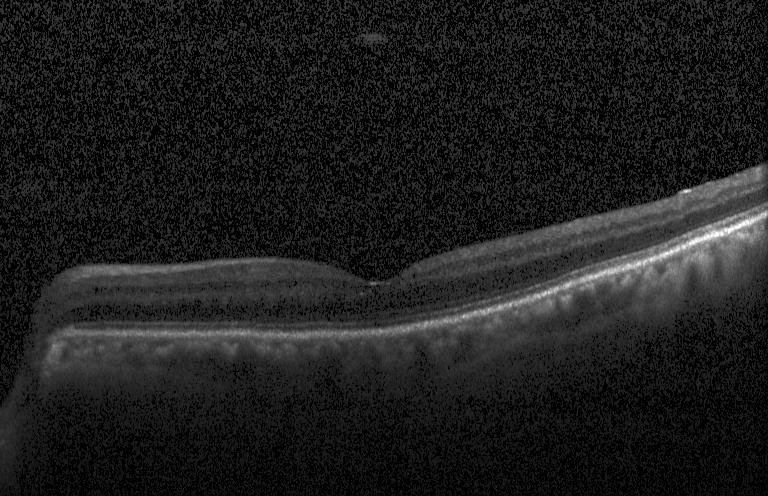 Optical coherence tomography scan · SD-OCT · centered on the fovea · acquired on a Heidelberg Spectralis. Assessment: no choroidal neovascularization, diabetic macular edema, or drusen.